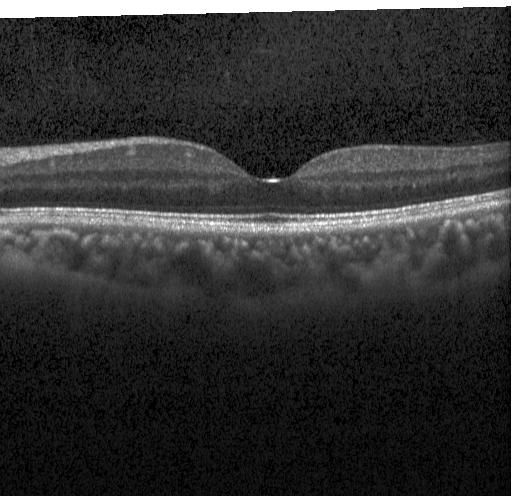

Heidelberg Spectralis · macular scan · retinal OCT cross-section — The scan shows no evidence of choroidal neovascularization, diabetic macular edema, or drusen.